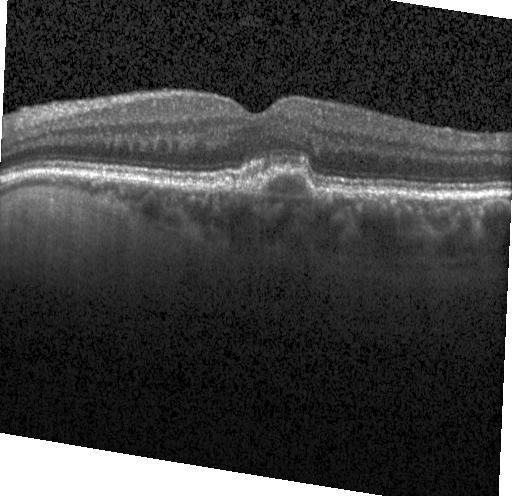

Dx: choroidal neovascularization.